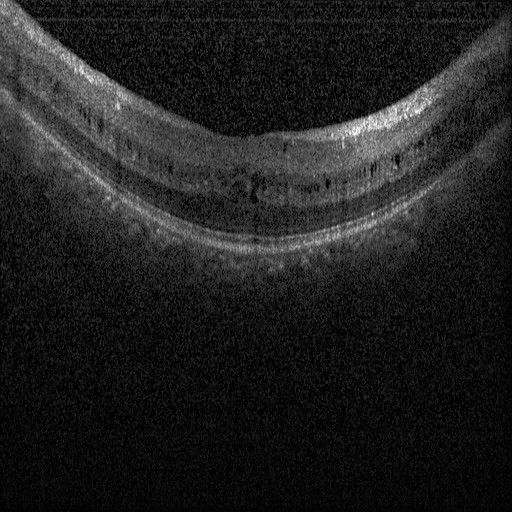

Dx: diabetic macular edema (DME).